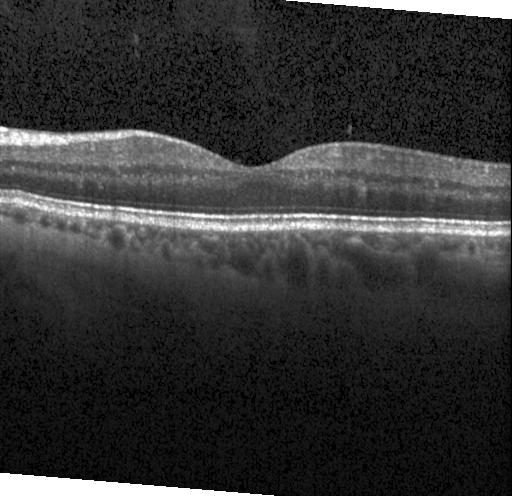

Optical coherence tomography scan, spectral-domain optical coherence tomography, Heidelberg Spectralis OCT system. Impression: no evidence of CNV, DME, or drusen.